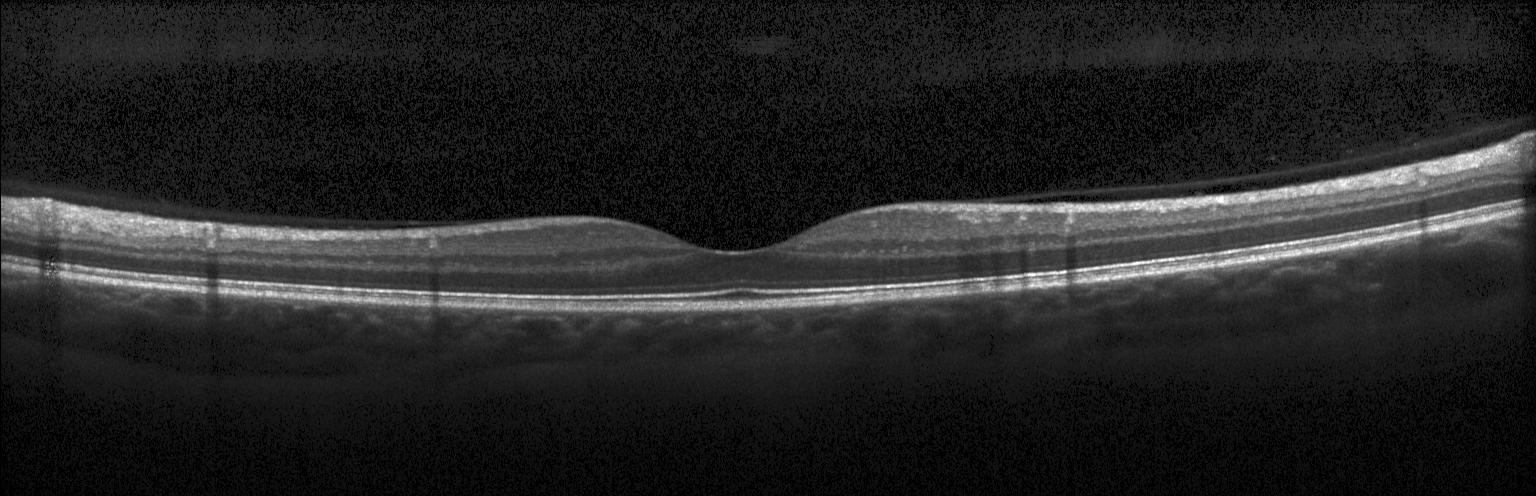

OCT line scan, spectral-domain OCT, centered on the fovea, Heidelberg Spectralis OCT system — Diagnosis: no CNV, DME, or drusen.